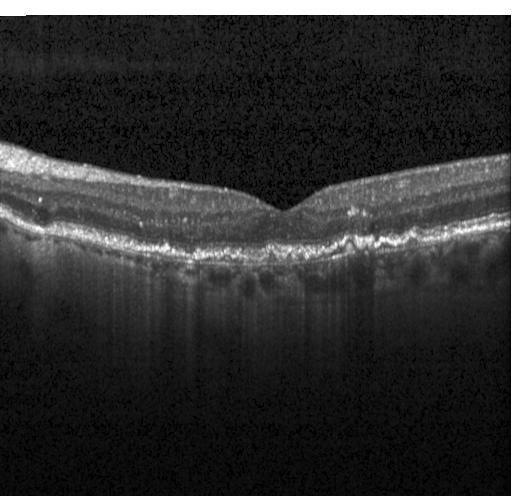
OCT finding: drusen.